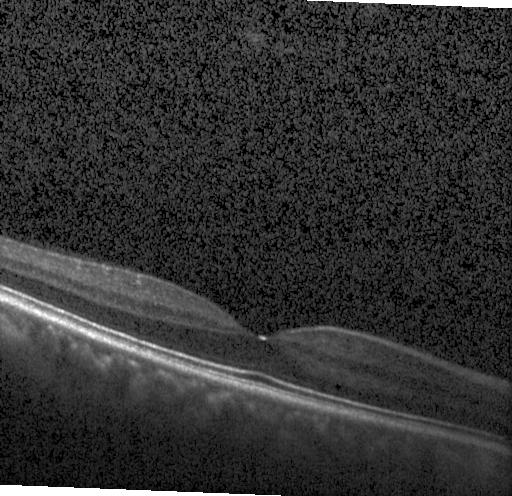 Instrument: Heidelberg Spectralis; macular scan; optical coherence tomography B-scan. This B-scan demonstrates no choroidal neovascularization, no diabetic macular edema, and no drusen.